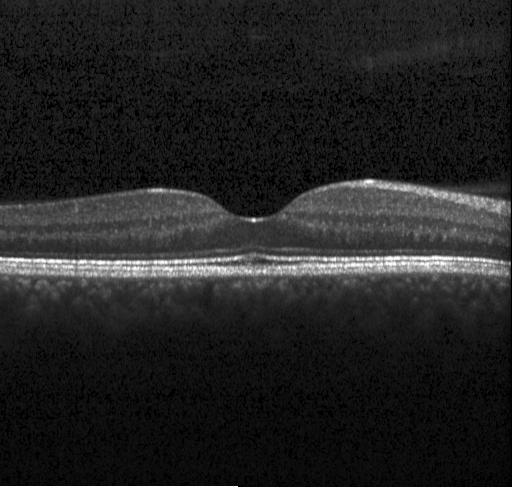 Heidelberg Spectralis. SD-OCT. Optical coherence tomography B-scan.
OCT finding: no choroidal neovascularization, no diabetic macular edema, and no drusen.